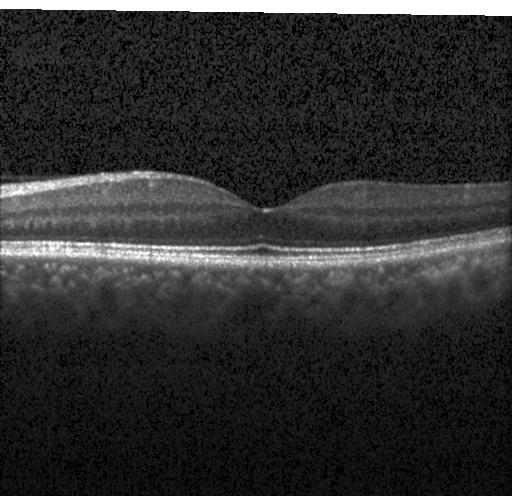 OCT line scan. This B-scan demonstrates neither choroidal neovascularization, diabetic macular edema, nor drusen.